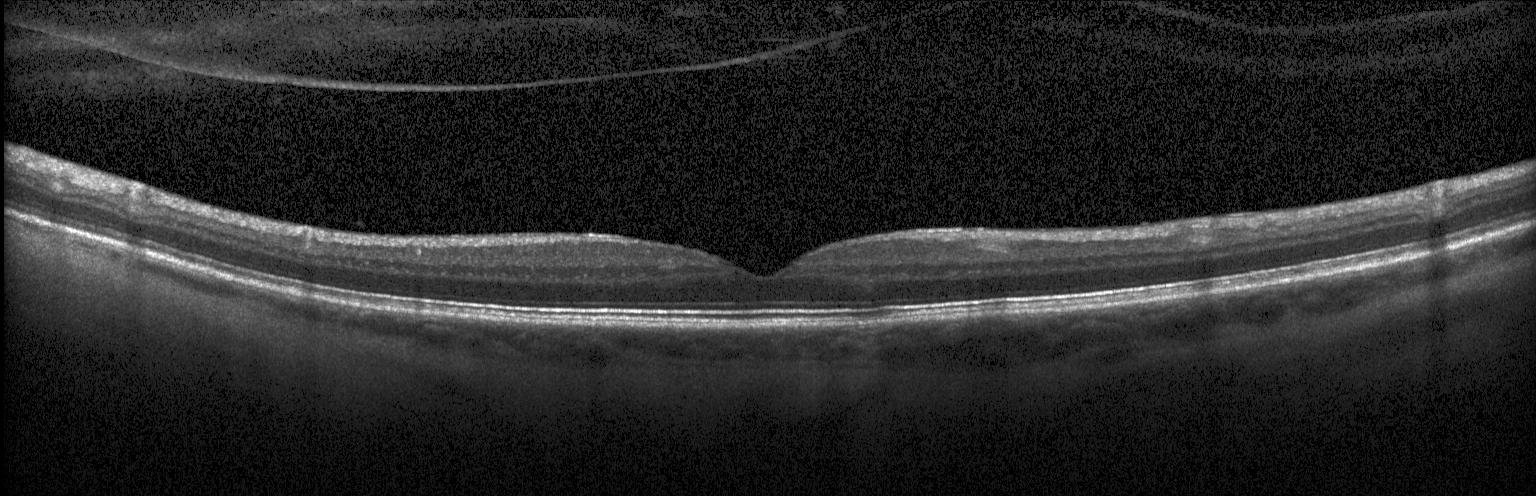

Retinal OCT B-scan — Finding: no evidence of choroidal neovascularization, diabetic macular edema, or drusen.